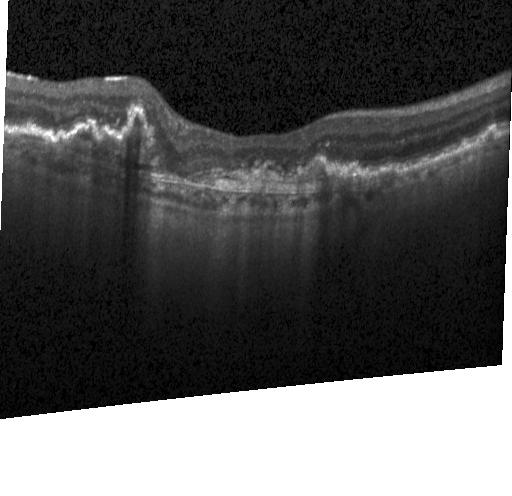
Macular OCT demonstrating a choroidal neovascular membrane.